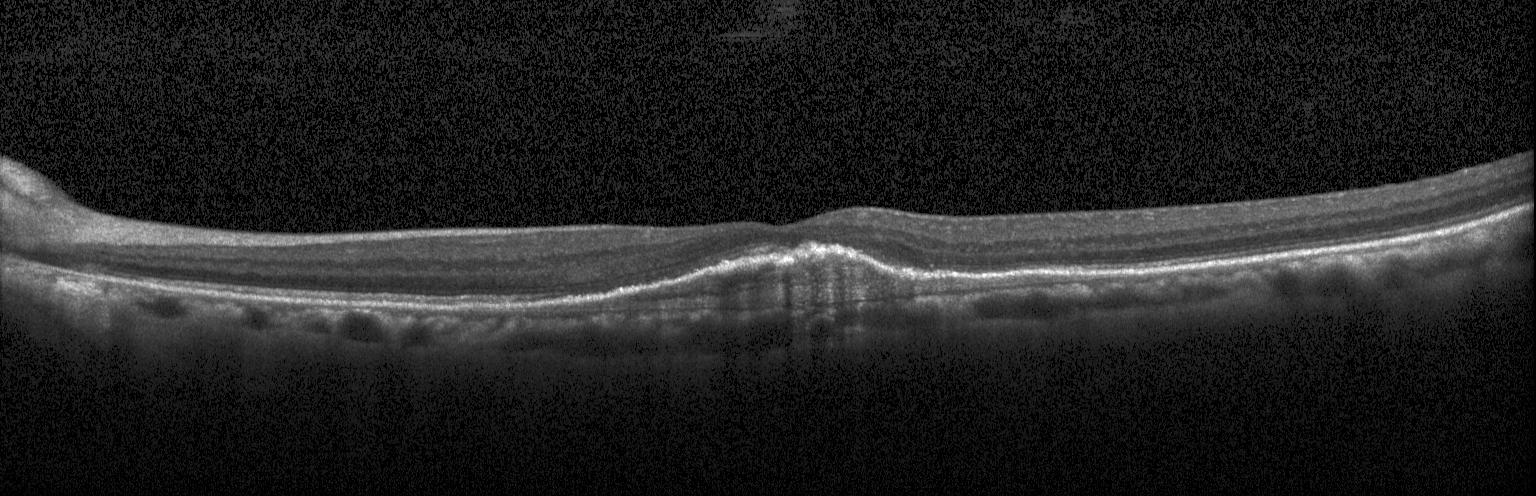 Impression: choroidal neovascularization (CNV).